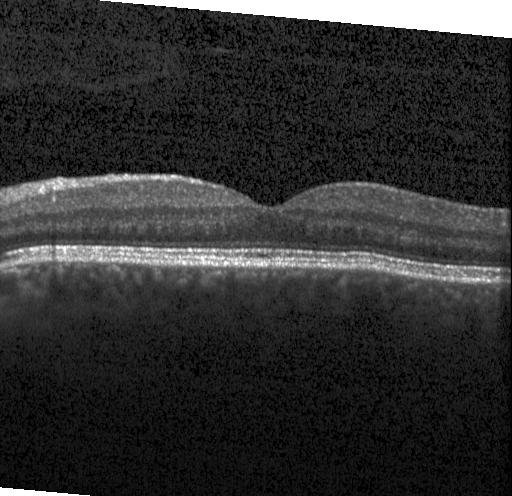 Through the macula, OCT line scan, spectral-domain OCT — Assessment: neither CNV, DME, nor drusen.